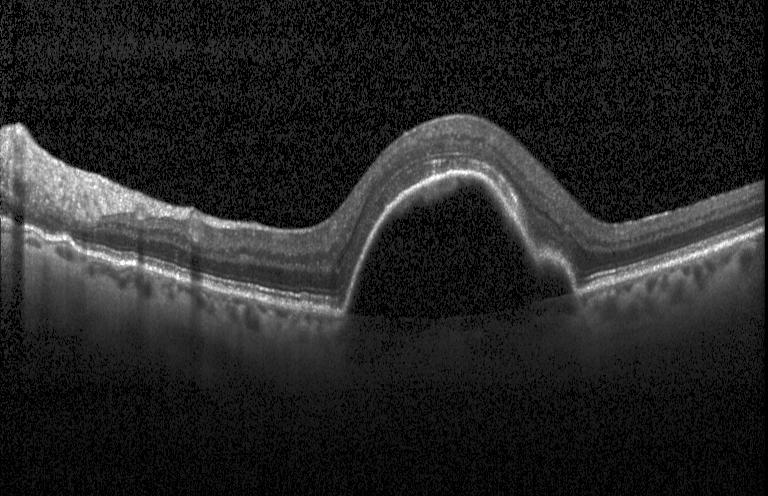

Fovea-centered · retinal OCT B-scan · Heidelberg Spectralis OCT system. Finding: choroidal neovascularization.